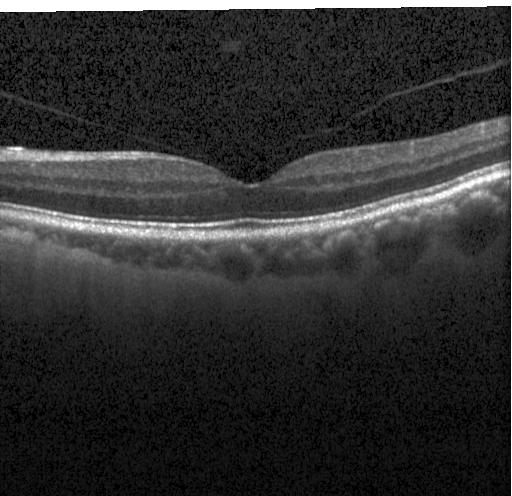 Dx: no evidence of CNV, DME, or drusen.